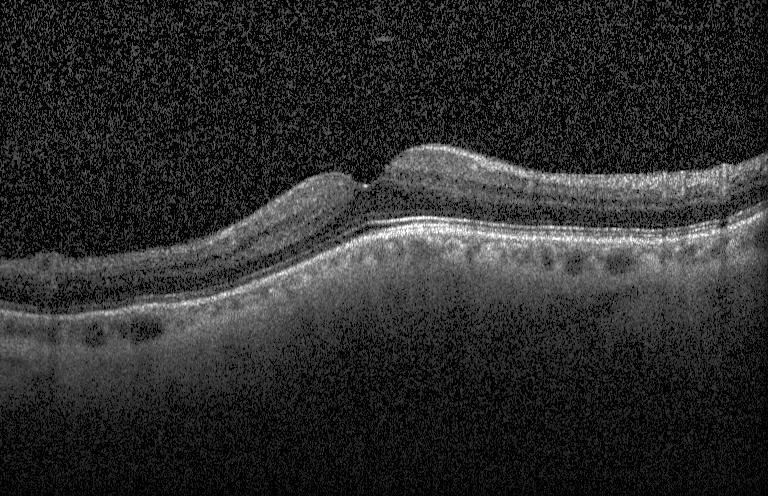

Heidelberg Spectralis OCT system, OCT B-scan, through the macula
Neither choroidal neovascularization, diabetic macular edema, nor drusen.